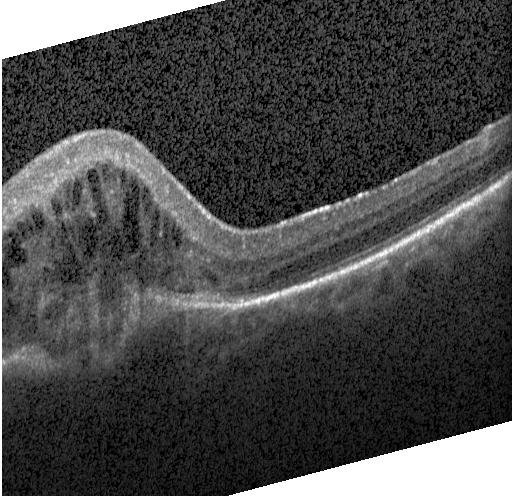

SD-OCT · retinal OCT cross-section.
Finding: a choroidal neovascular membrane.